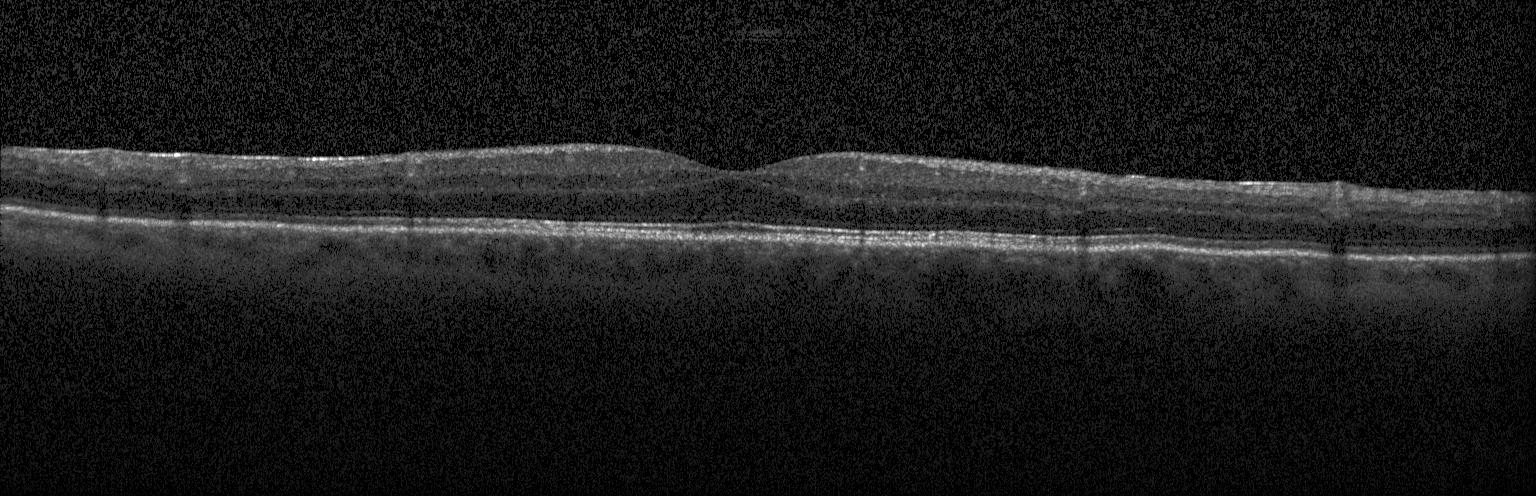 Through the macula, OCT line scan — Diagnosis: no evidence of choroidal neovascularization, diabetic macular edema, or drusen.